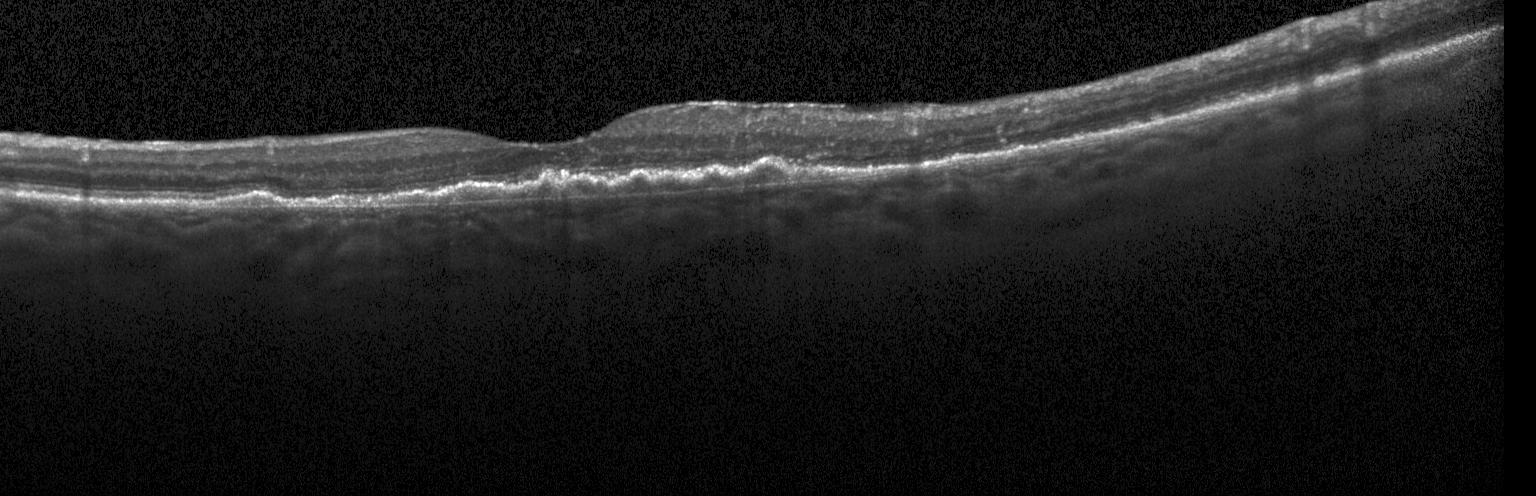 Instrument: Heidelberg Spectralis, retinal OCT B-scan, spectral-domain OCT.
Finding: choroidal neovascularization (CNV).